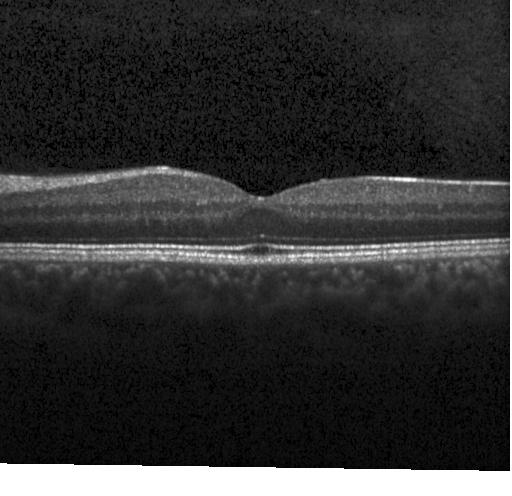 Retinal OCT cross-section showing no evidence of CNV, DME, or drusen.